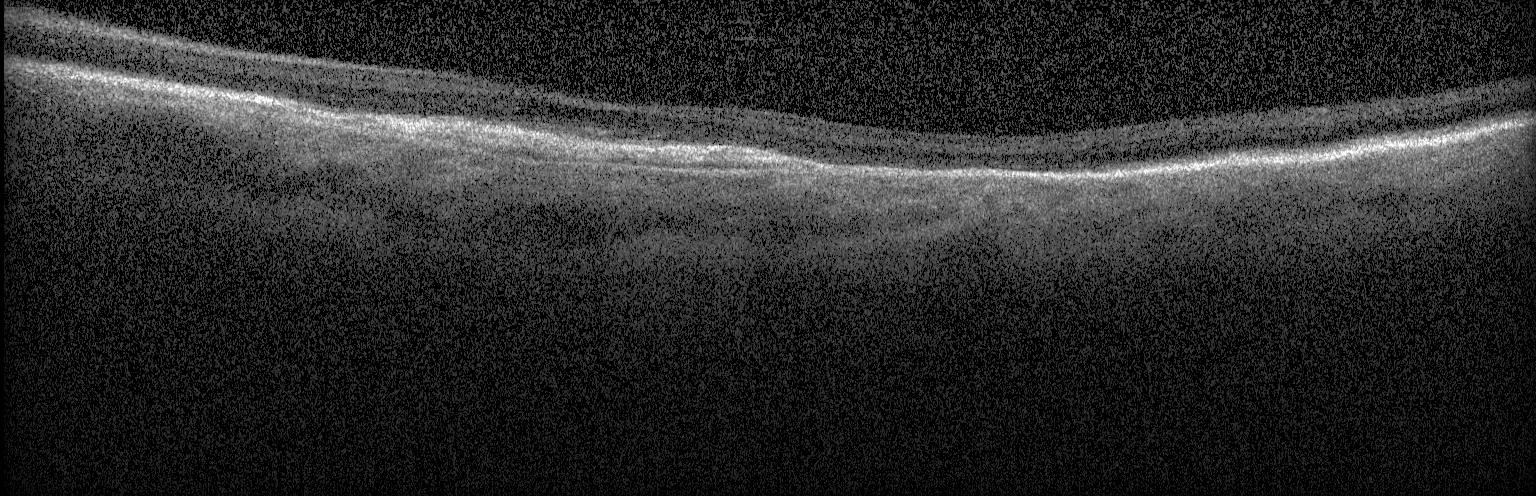
OCT line scan. Spectral-domain OCT. Through the macula.
Assessment: a choroidal neovascular membrane.